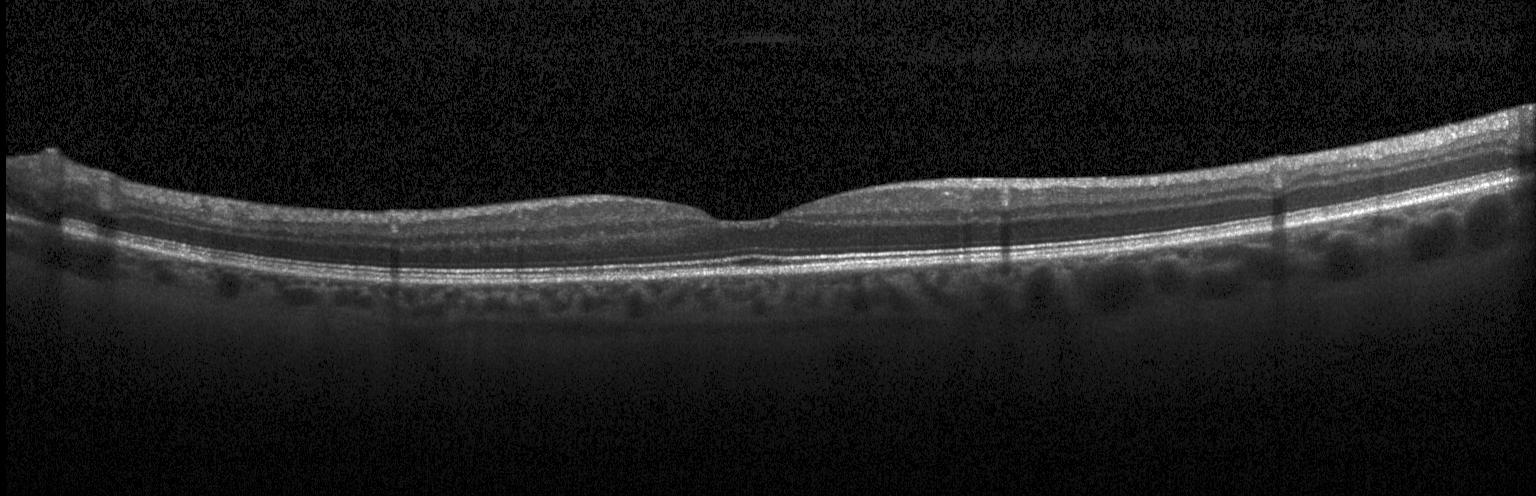 Retinal OCT cross-section, acquired on a Heidelberg Spectralis, SD-OCT. Impression: no evidence of choroidal neovascularization, diabetic macular edema, or drusen.